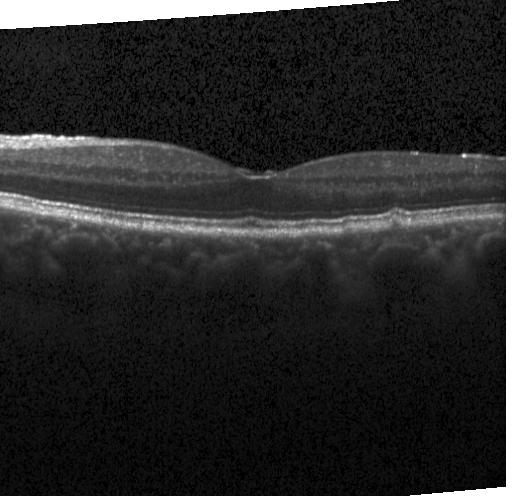
Impression: multiple drusen.